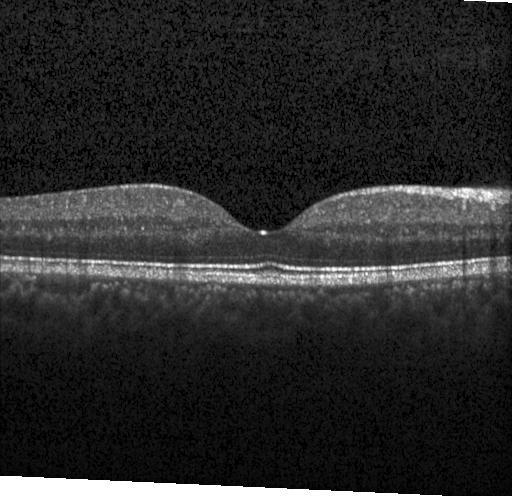 Retinal OCT cross-section.
Macular OCT: no choroidal neovascularization, no diabetic macular edema, and no drusen.